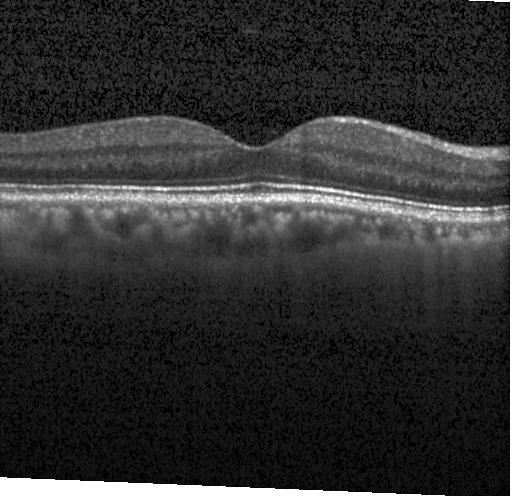

Optical coherence tomography B-scan.
Dx: neither choroidal neovascularization, diabetic macular edema, nor drusen.